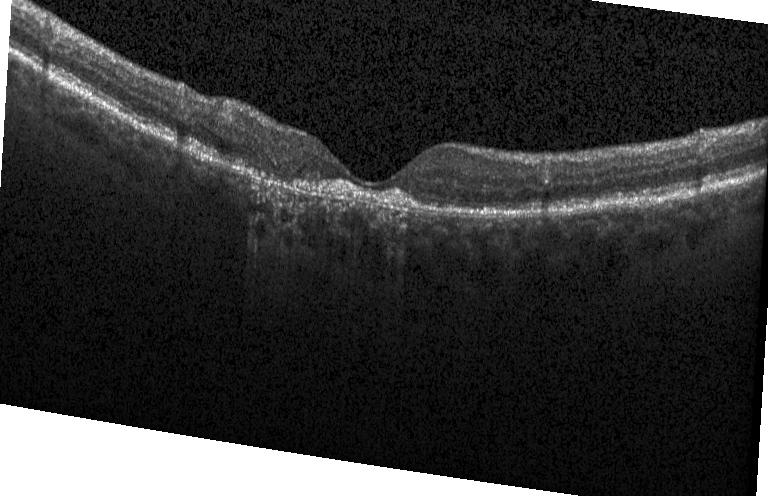
Heidelberg Spectralis OCT system · OCT B-scan · spectral-domain optical coherence tomography
Impression: a choroidal neovascular membrane.